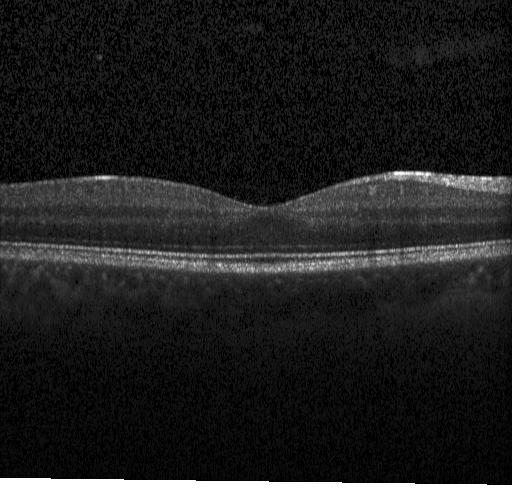
OCT B-scan showing no evidence of choroidal neovascularization, diabetic macular edema, or drusen.